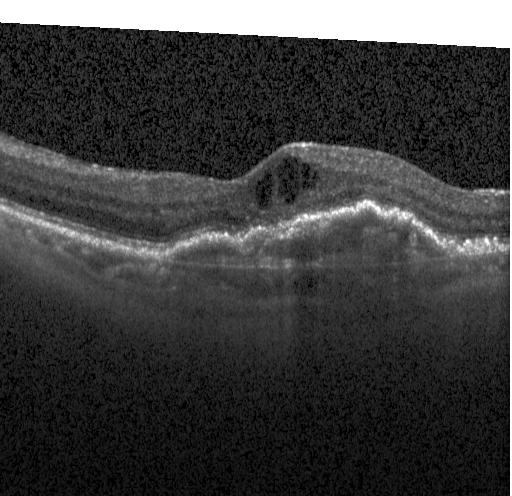
Optical coherence tomography scan · Heidelberg Spectralis.
Choroidal neovascularization.